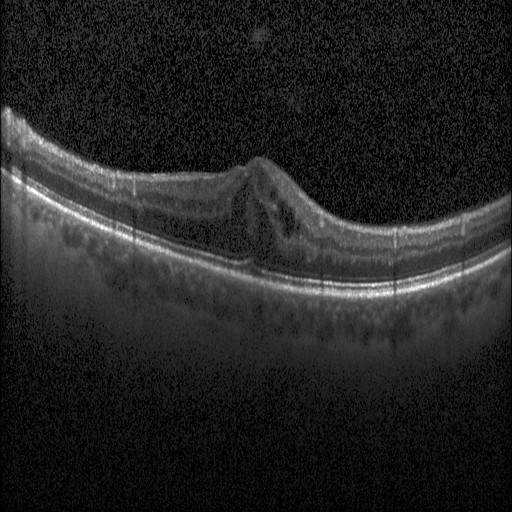

Retinal OCT cross-section.
This B-scan demonstrates diabetic macular edema.